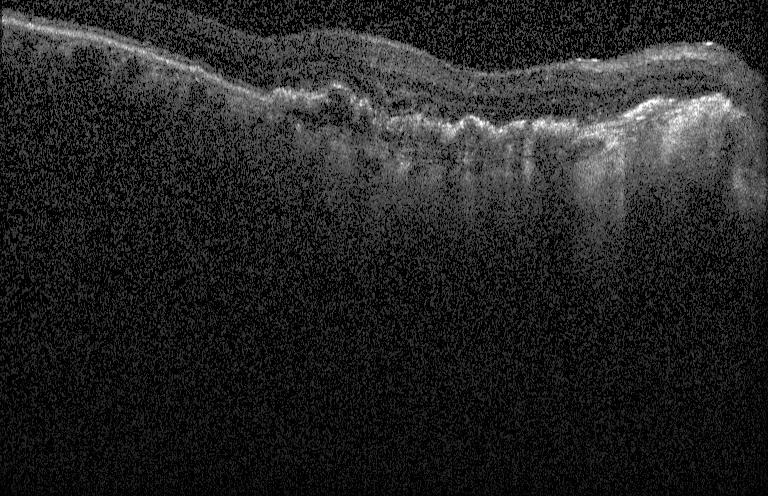 OCT B-scan; spectral-domain OCT.
Impression: a choroidal neovascular membrane.